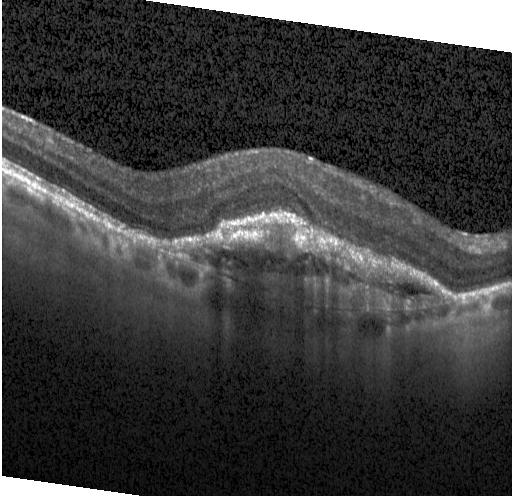

Acquired on a Heidelberg Spectralis; optical coherence tomography scan; SD-OCT.
A choroidal neovascular membrane.